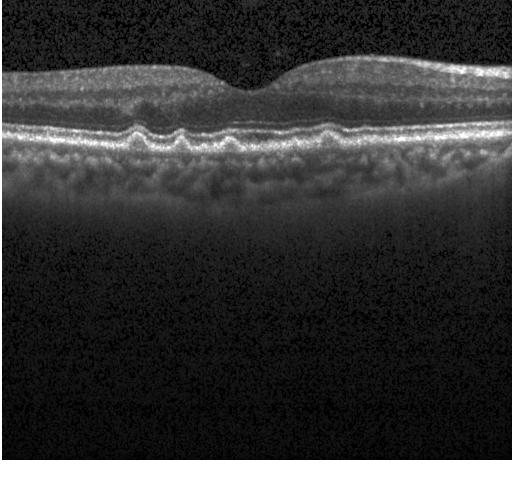
Retinal OCT cross-section; through the macula. This B-scan demonstrates drusen.